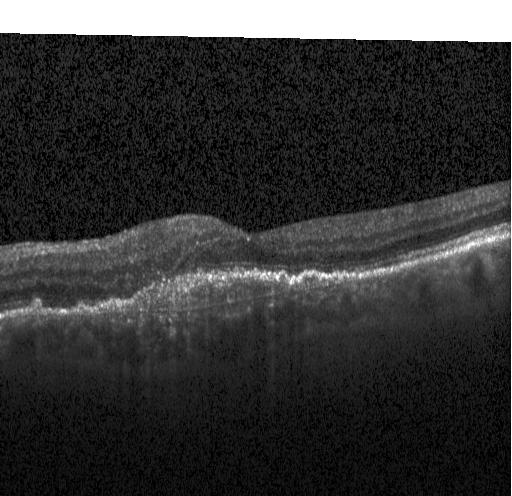

Through the macula · OCT B-scan · spectral-domain OCT · Heidelberg Spectralis.
A choroidal neovascular membrane.